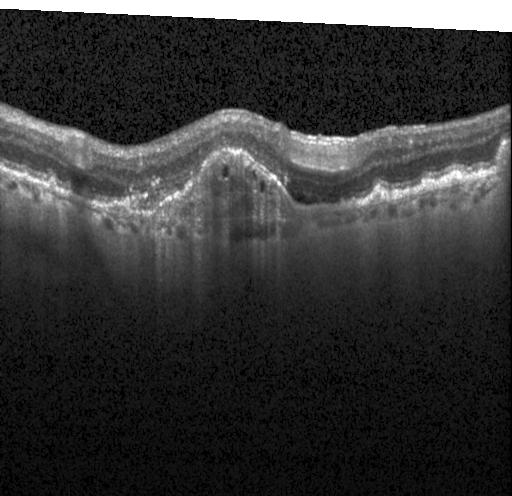

Diagnosis: choroidal neovascularization.